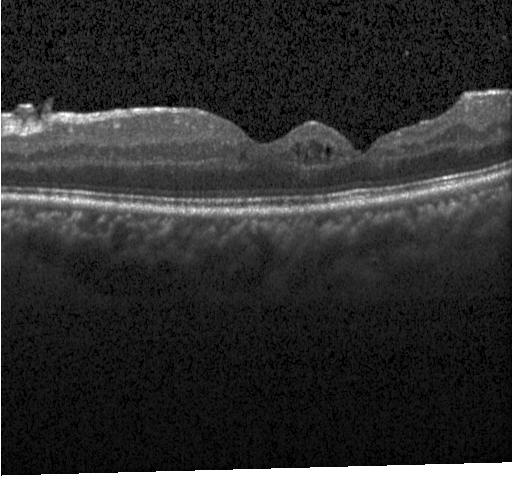
Diagnosis: diabetic macular edema.